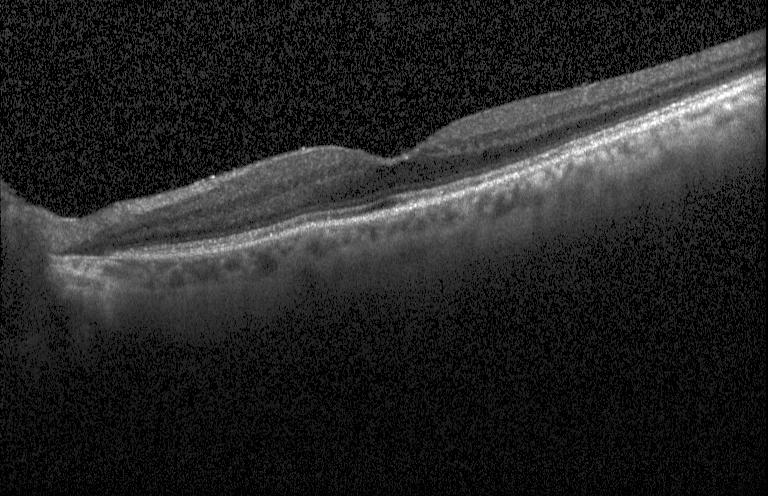

Retinal OCT B-scan. Heidelberg Spectralis OCT system. Spectral-domain optical coherence tomography. Fovea-centered — Finding: no choroidal neovascularization, no diabetic macular edema, and no drusen.